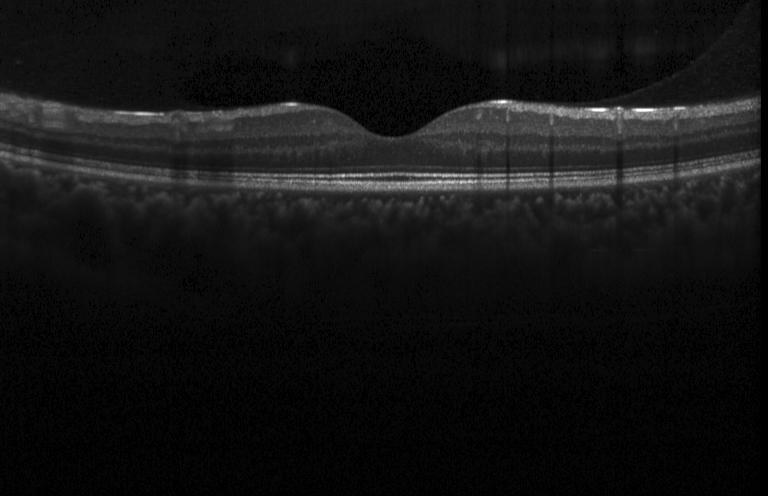 Dx: no CNV, DME, or drusen.